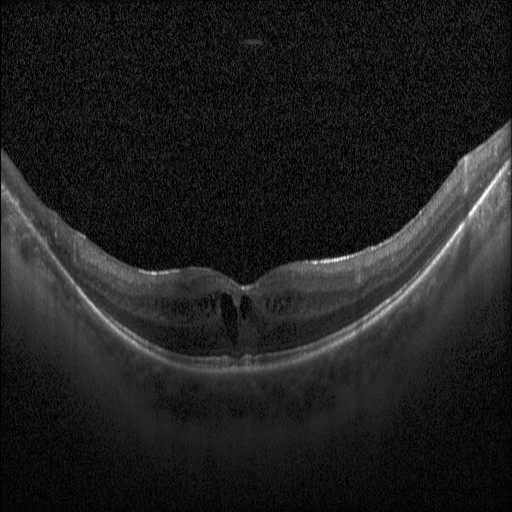 Spectral-domain optical coherence tomography · retinal OCT cross-section — OCT finding: DME.